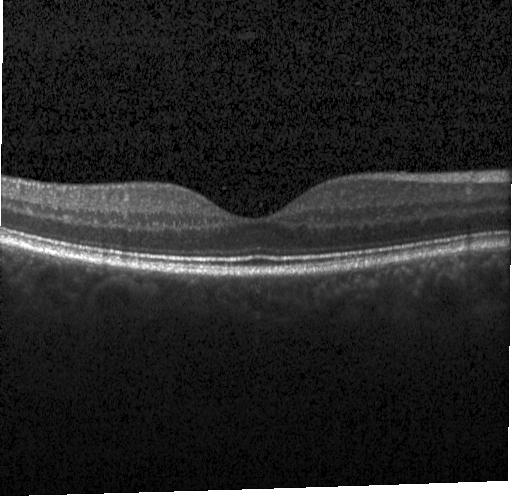

SD-OCT · retinal OCT cross-section · horizontal scan through the fovea.
The scan shows neither choroidal neovascularization, diabetic macular edema, nor drusen.